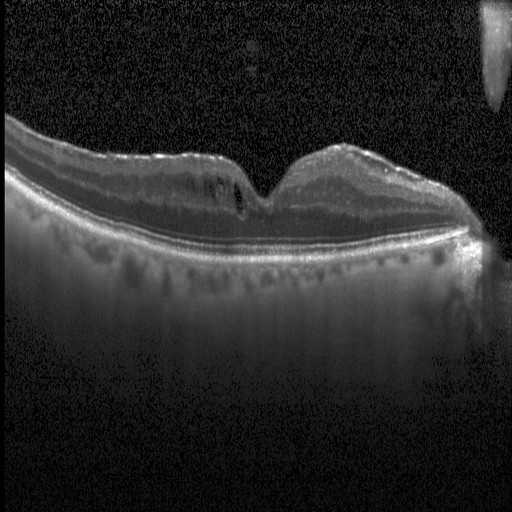
OCT finding: DME.